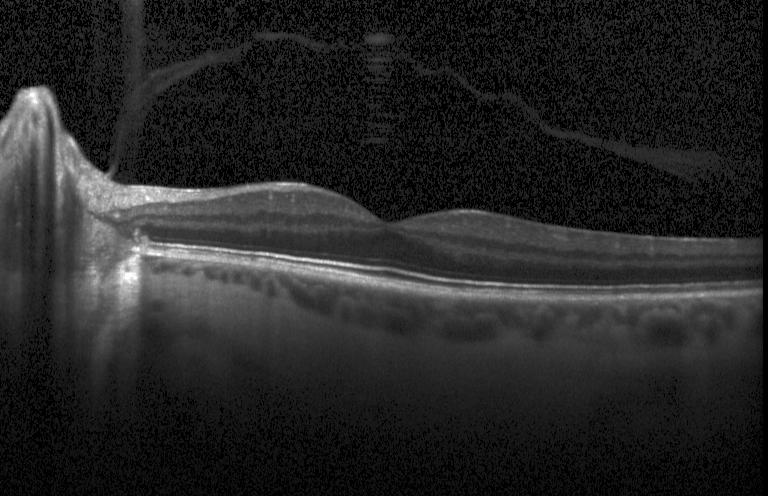 Impression: no choroidal neovascularization, diabetic macular edema, or drusen.